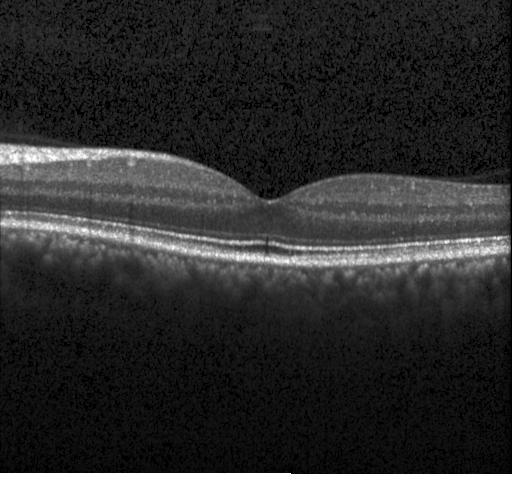
Optical coherence tomography B-scan
Impression: neither choroidal neovascularization, diabetic macular edema, nor drusen.